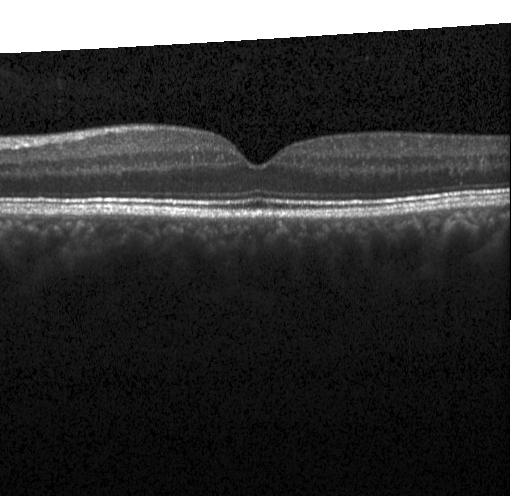

Acquired on a Heidelberg Spectralis. SD-OCT. OCT B-scan.
Assessment: neither choroidal neovascularization, diabetic macular edema, nor drusen.